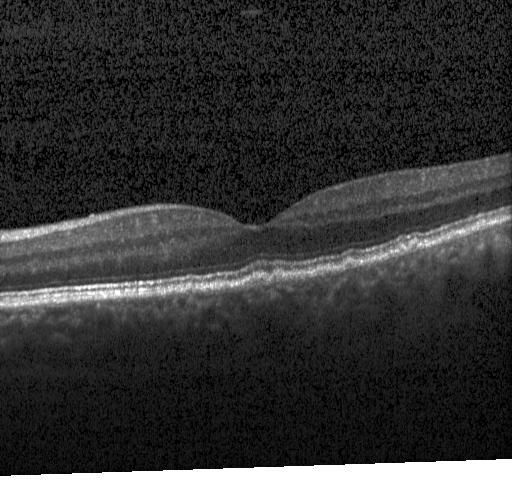 Retinal OCT cross-section — The scan shows drusen.